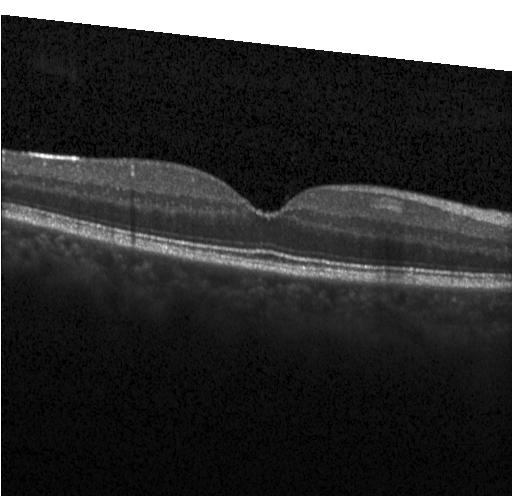

Diagnosis: no evidence of choroidal neovascularization, diabetic macular edema, or drusen.